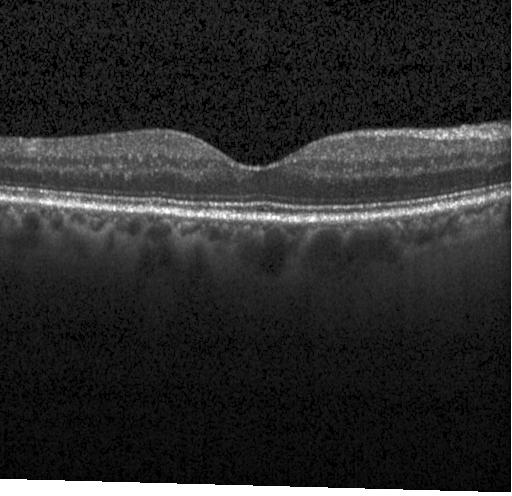

OCT B-scan · macular scan
Finding: no evidence of choroidal neovascularization, diabetic macular edema, or drusen.